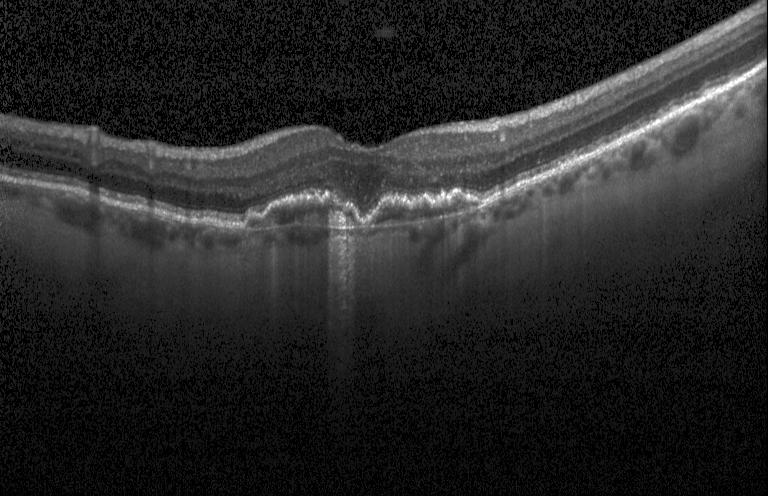
Retinal OCT cross-section showing choroidal neovascularization.